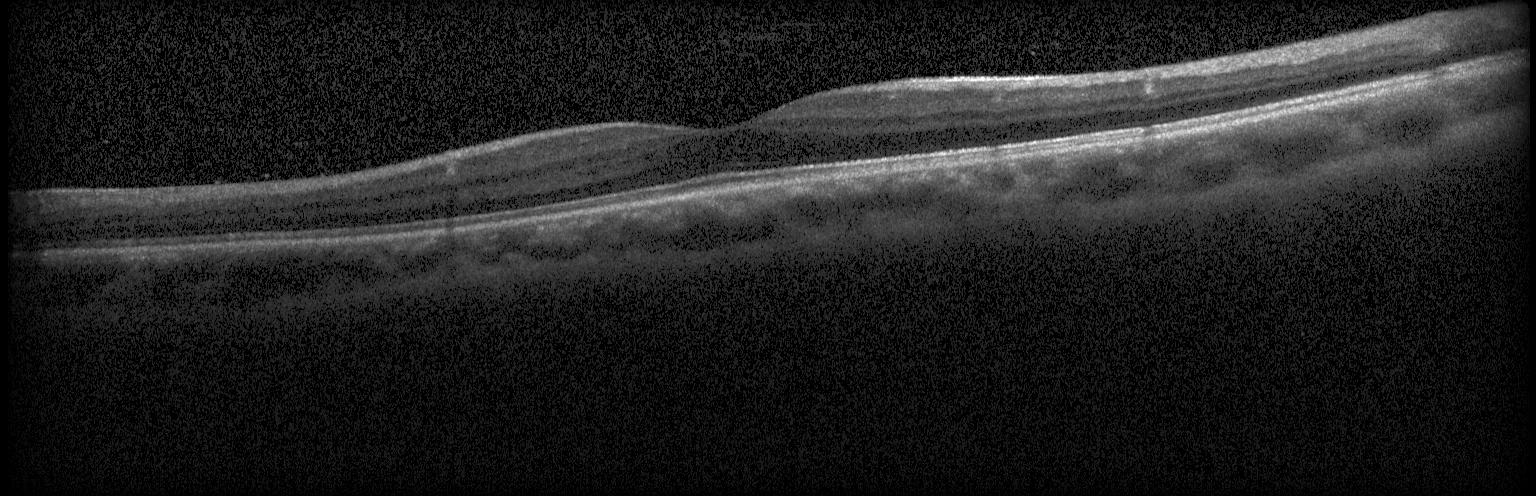
OCT finding: neither choroidal neovascularization, diabetic macular edema, nor drusen.